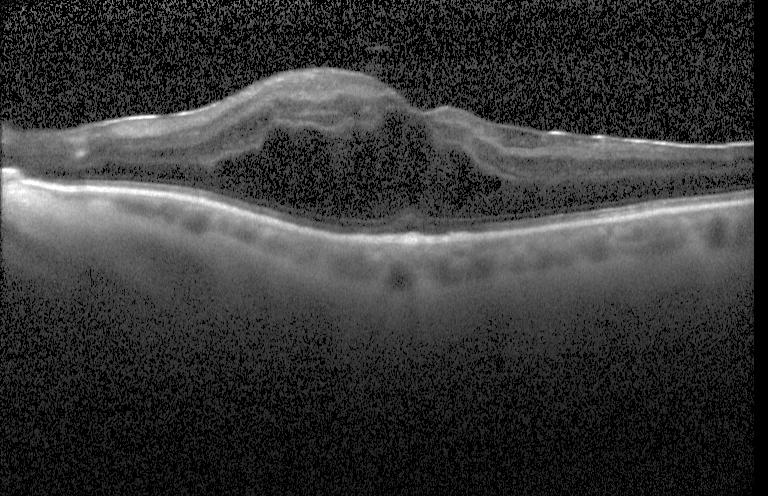 Optical coherence tomography scan; SD-OCT. Finding: diabetic macular edema.